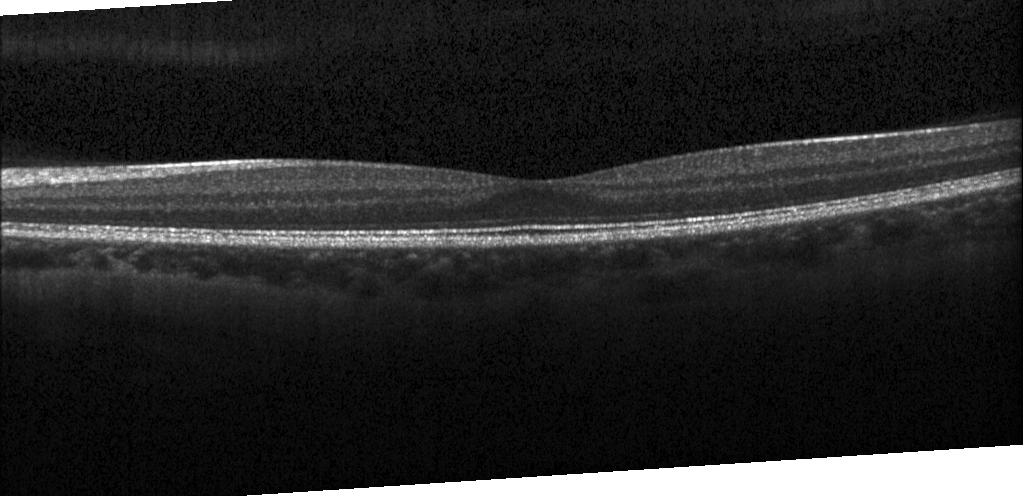 Spectral-domain optical coherence tomography; Heidelberg Spectralis; retinal OCT cross-section; fovea-centered
Diagnosis: neither choroidal neovascularization, diabetic macular edema, nor drusen.